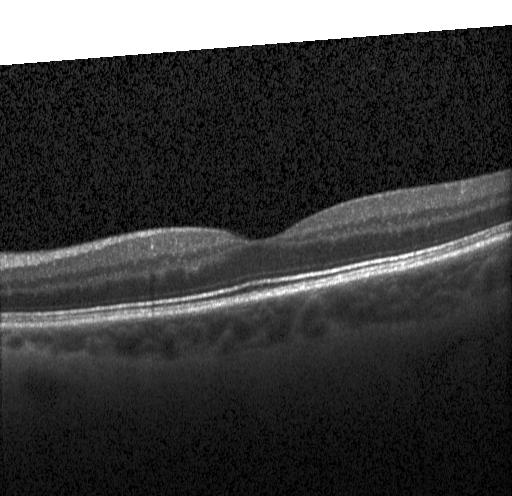 Diagnosis: neither choroidal neovascularization, diabetic macular edema, nor drusen.